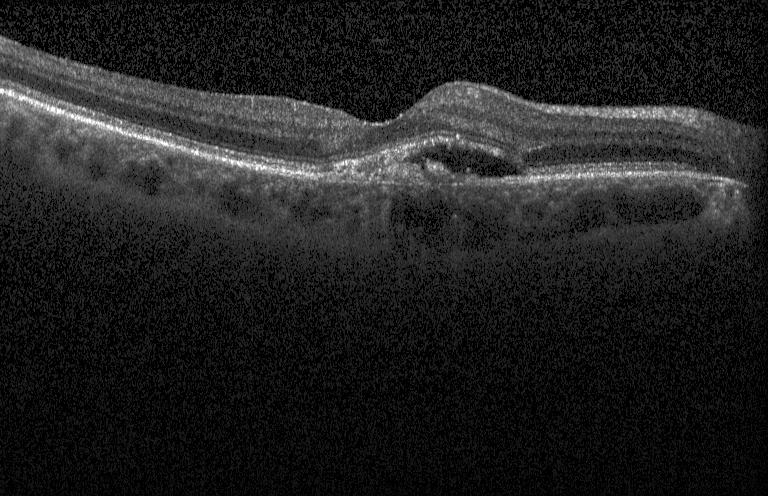
Optical coherence tomography B-scan; centered on the fovea. This B-scan demonstrates choroidal neovascularization.